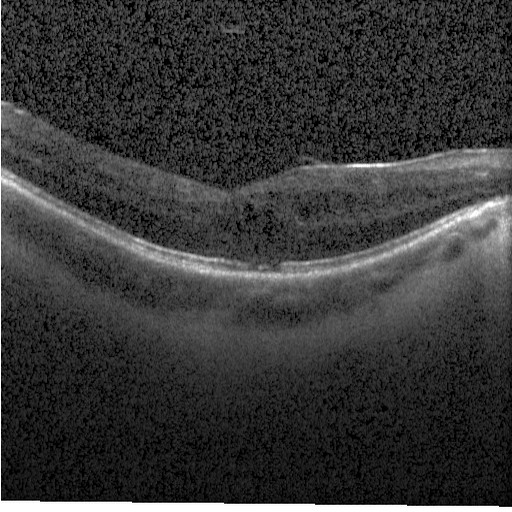

SD-OCT · OCT line scan.
This B-scan demonstrates diabetic macular edema (DME).